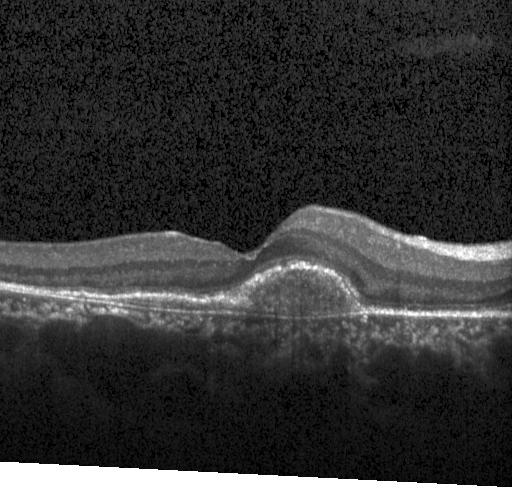

OCT line scan.
Dx: choroidal neovascularization.